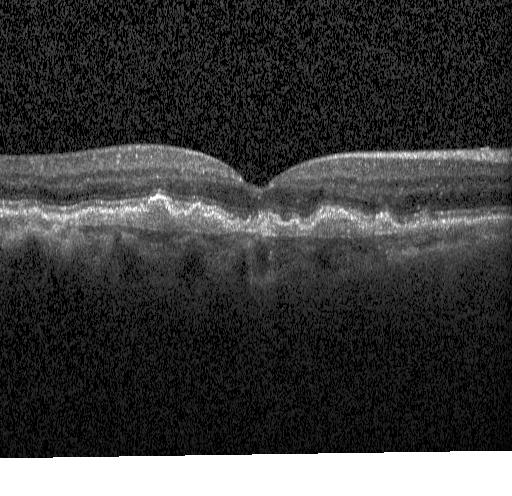
A choroidal neovascular membrane.